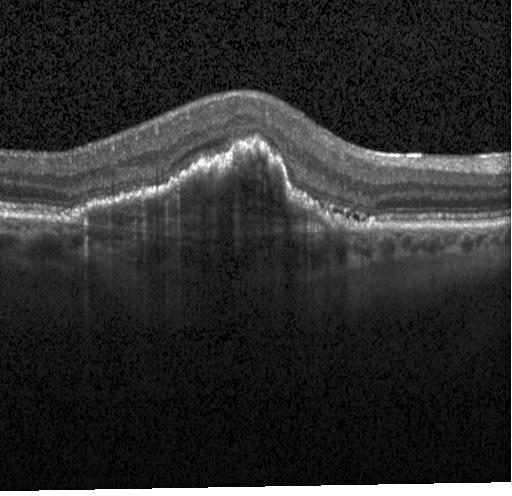
This B-scan demonstrates a choroidal neovascular membrane.